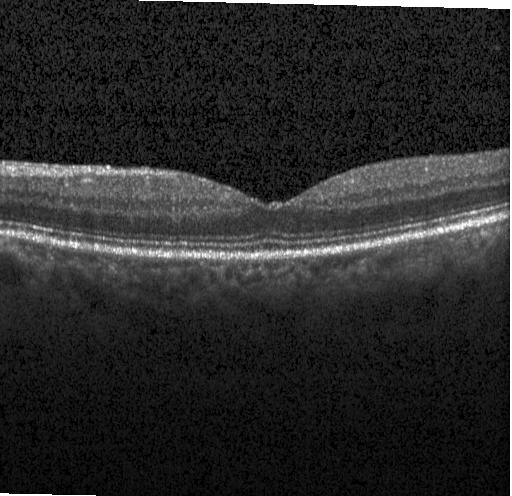

The scan shows no evidence of choroidal neovascularization, diabetic macular edema, or drusen.